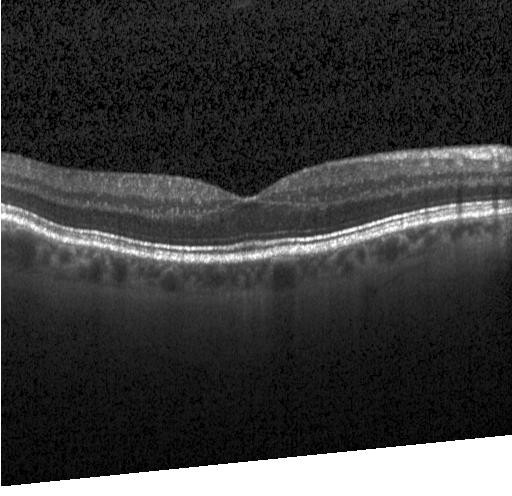
Optical coherence tomography scan; macular scan. Finding: no evidence of CNV, DME, or drusen.